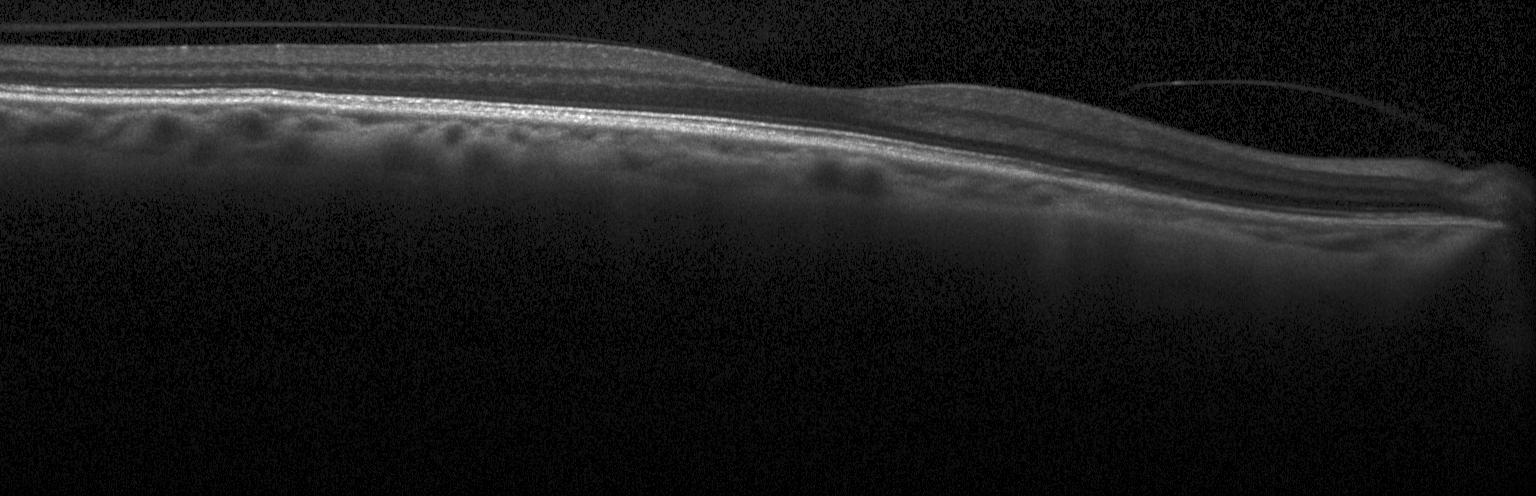
Diagnosis: no evidence of choroidal neovascularization, diabetic macular edema, or drusen.